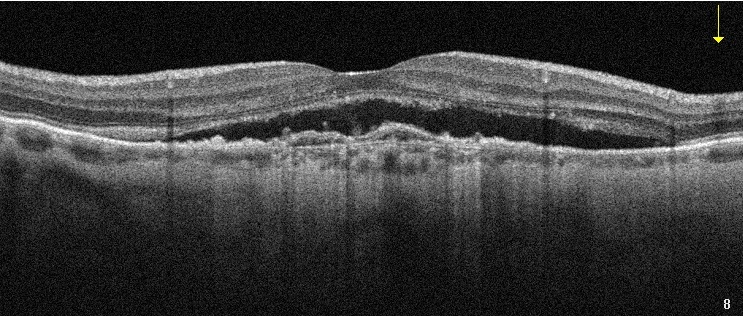
Optovue Avanti RTVue XR. Retinal OCT cross-section — Impression: age-related macular degeneration (AMD).